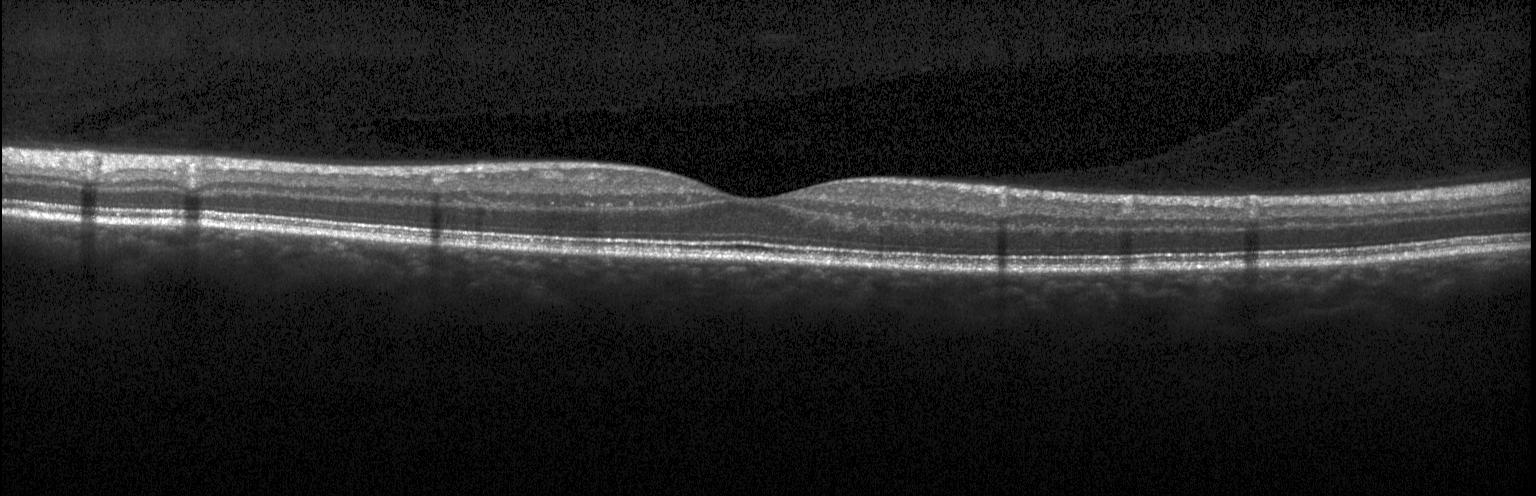
Instrument: Heidelberg Spectralis · retinal OCT B-scan · spectral-domain optical coherence tomography · through the macula — Finding: neither choroidal neovascularization, diabetic macular edema, nor drusen.